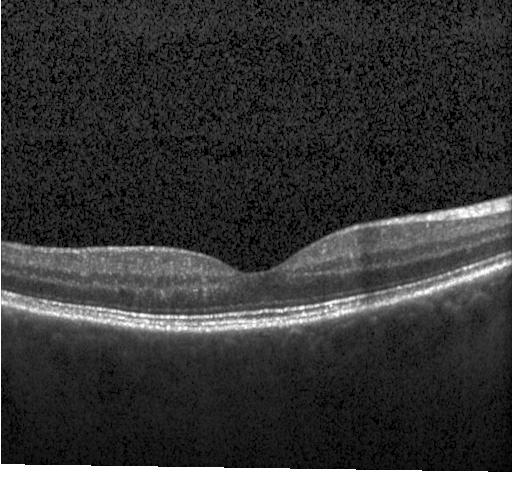

OCT finding: no choroidal neovascularization, diabetic macular edema, or drusen.